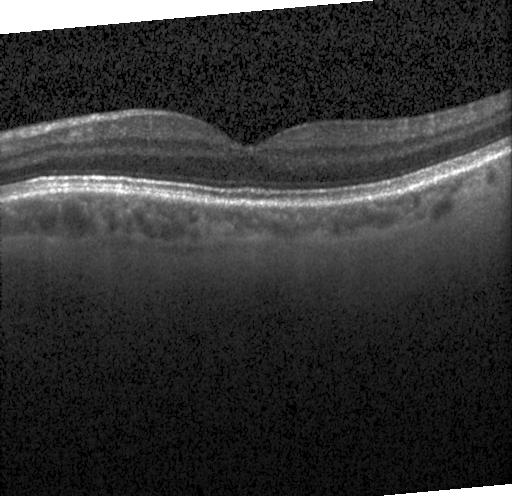
OCT line scan — The scan shows neither choroidal neovascularization, diabetic macular edema, nor drusen.